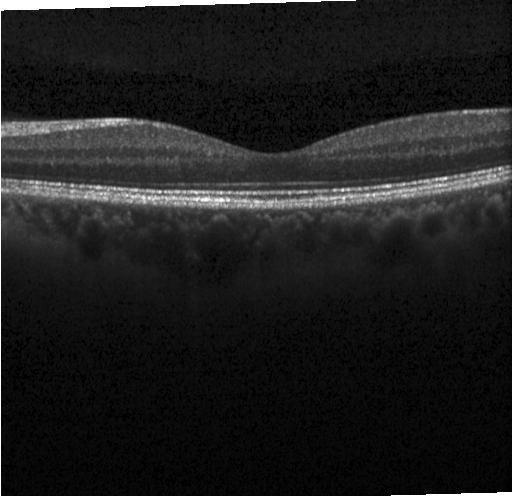

Impression: no choroidal neovascularization, diabetic macular edema, or drusen.